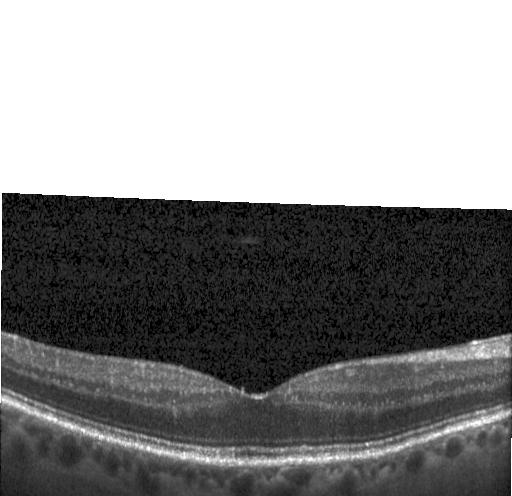

Diagnosis: no choroidal neovascularization, no diabetic macular edema, and no drusen.